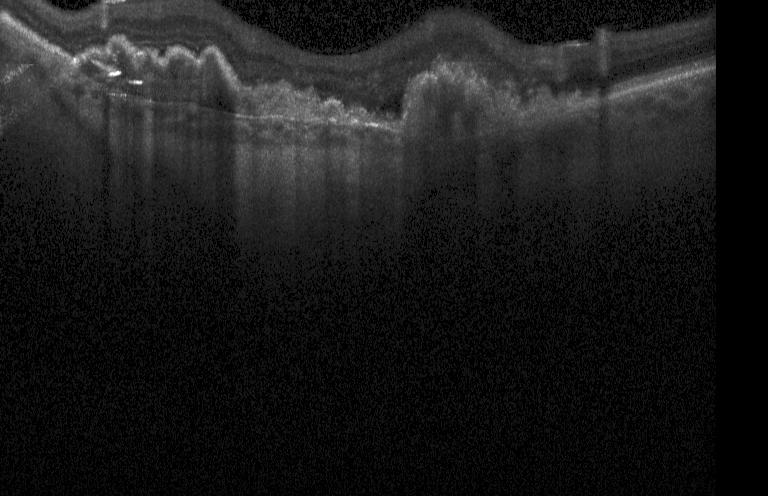 Optical coherence tomography scan. Impression: choroidal neovascularization.